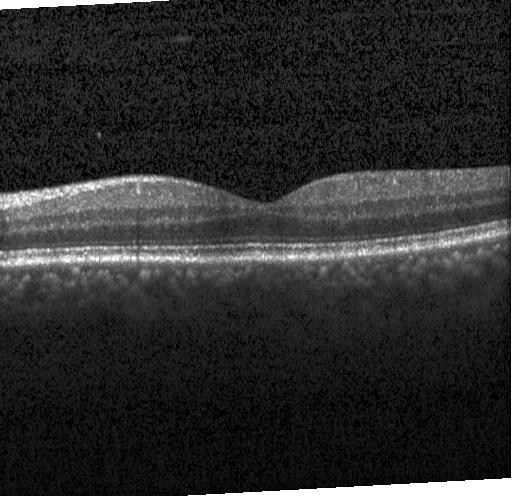 Diagnosis: no choroidal neovascularization, no diabetic macular edema, and no drusen.